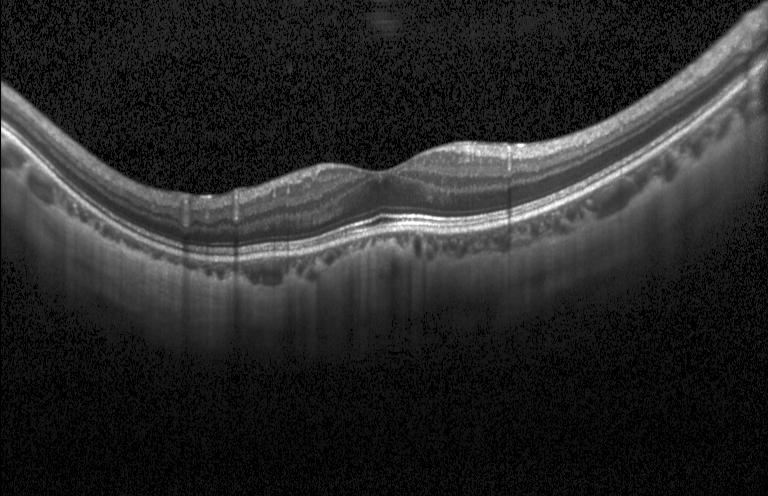
Heidelberg Spectralis. Centered on the fovea. OCT line scan
This B-scan demonstrates no choroidal neovascularization, no diabetic macular edema, and no drusen.